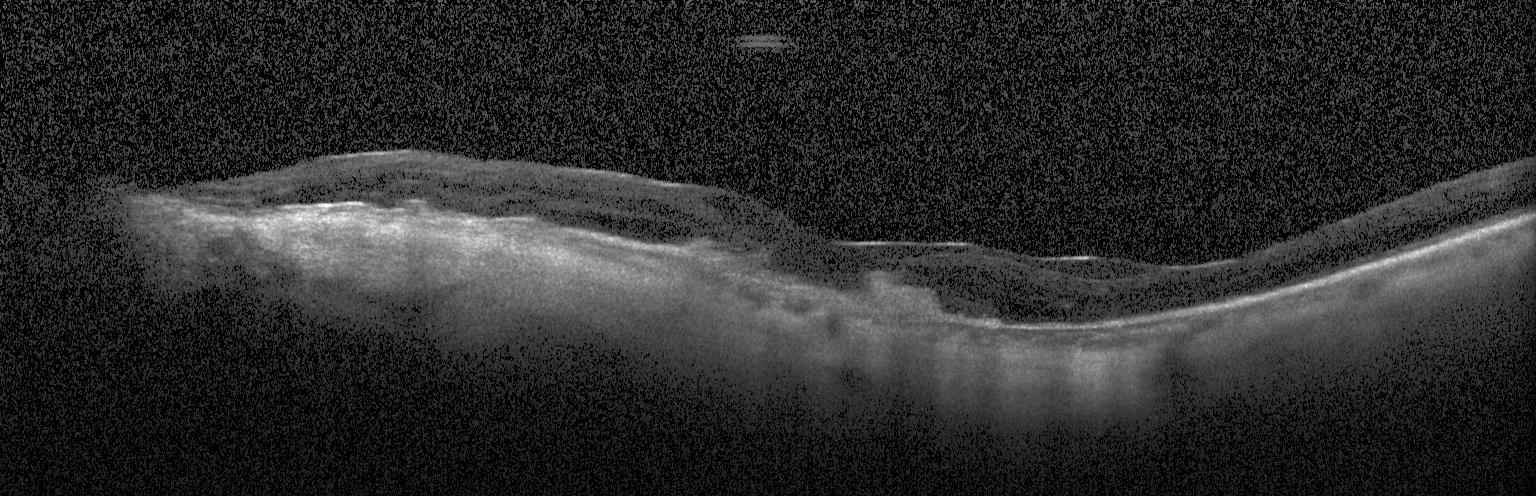 OCT finding: choroidal neovascularization.